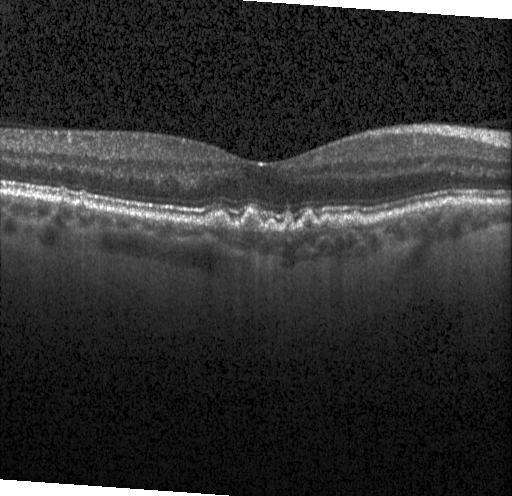
Optical coherence tomography scan; fovea-centered; instrument: Heidelberg Spectralis; spectral-domain optical coherence tomography
Impression: sub-RPE drusenoid deposits.